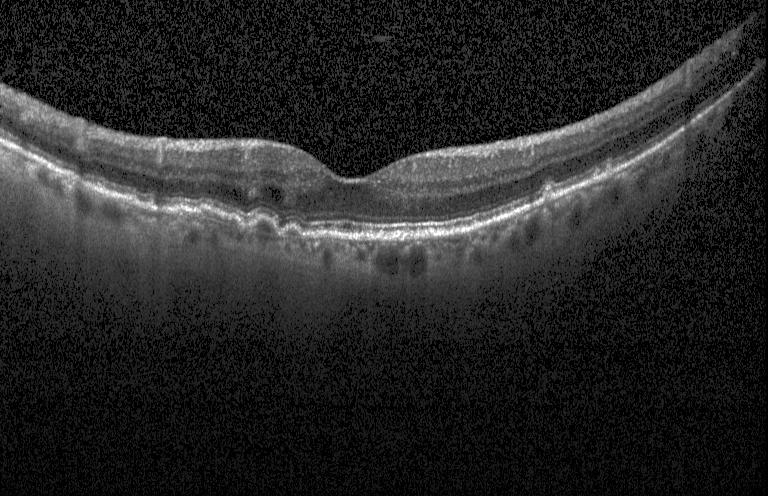

Assessment: multiple drusen.